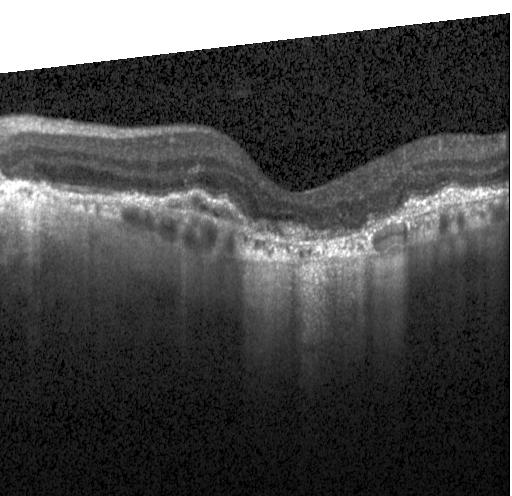 Diagnosis: choroidal neovascularization (CNV).